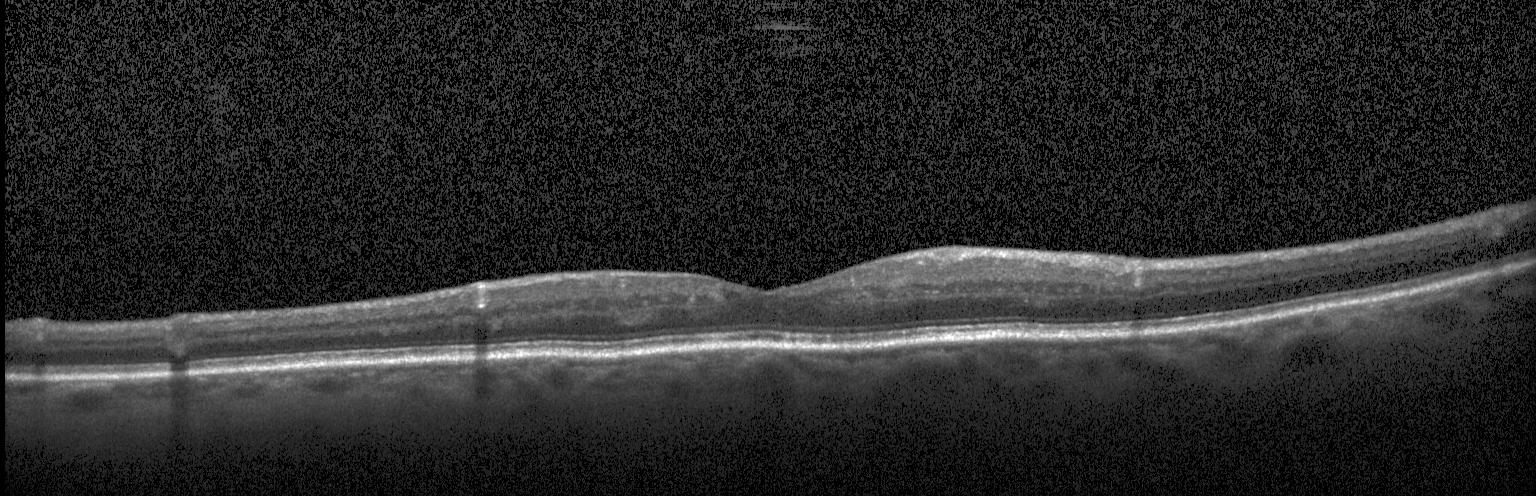
Optical coherence tomography scan · SD-OCT · centered on the fovea
Macular OCT: no evidence of choroidal neovascularization, diabetic macular edema, or drusen.